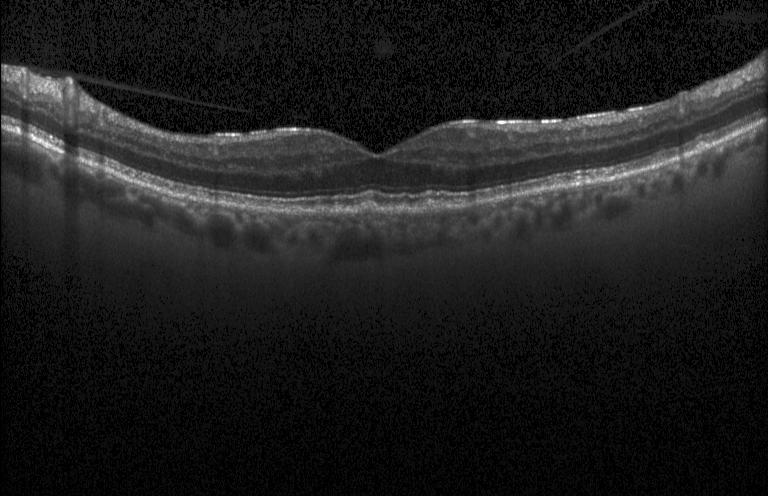 Diagnosis: sub-RPE drusenoid deposits.